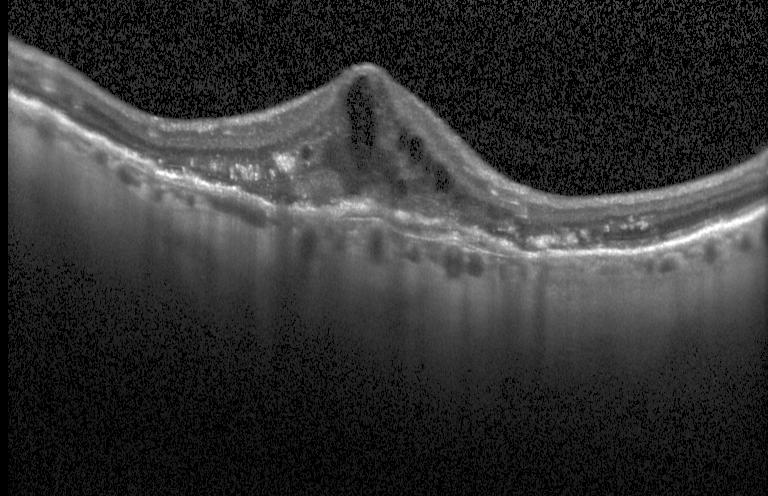

Optical coherence tomography scan; through the macula.
OCT finding: a choroidal neovascular membrane.